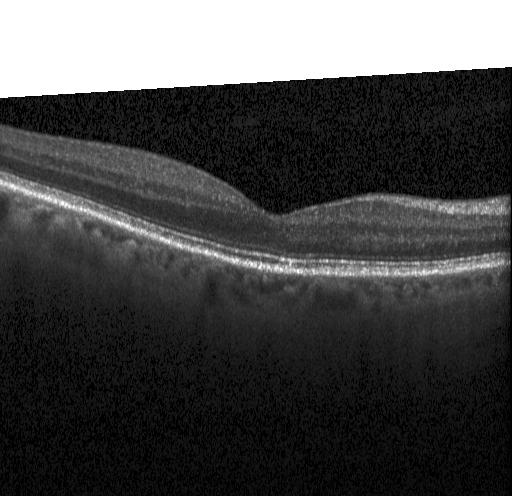 Retinal OCT cross-section.
Dx: no choroidal neovascularization, no diabetic macular edema, and no drusen.